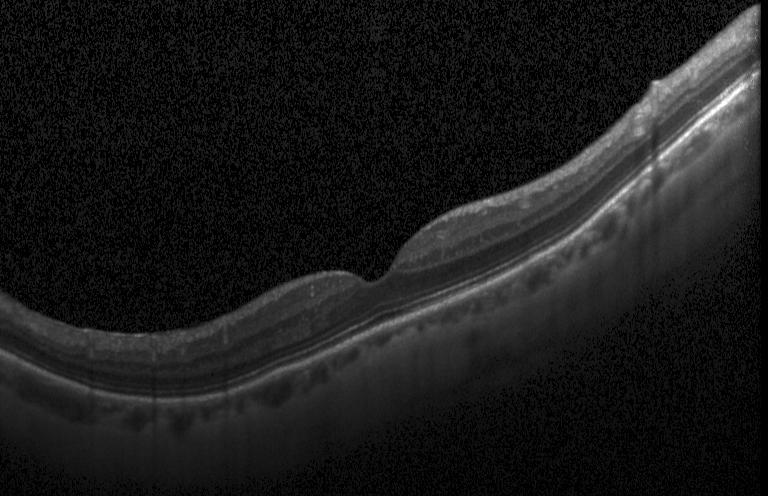 Diagnosis: no CNV, no DME, and no drusen.